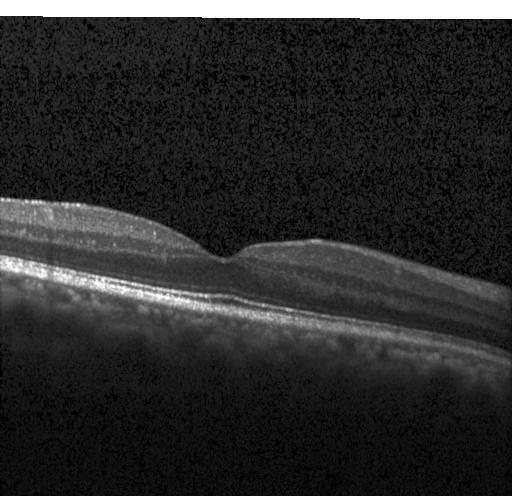

The scan shows no CNV, no DME, and no drusen.